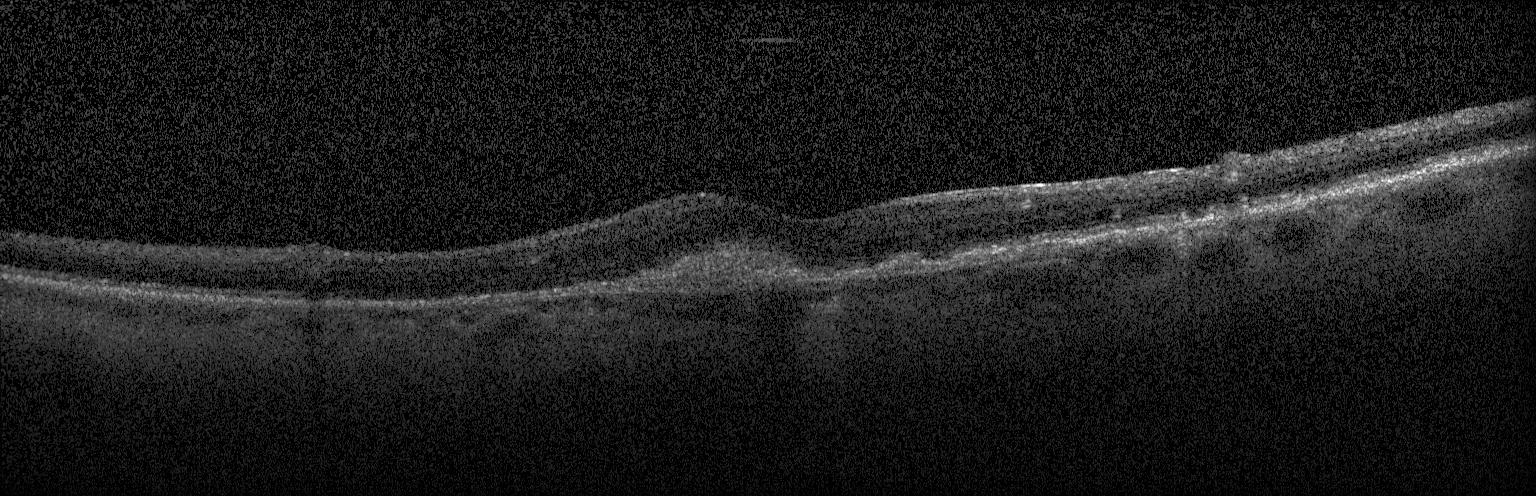

Instrument: Heidelberg Spectralis; spectral-domain OCT; through the macula; OCT B-scan — Assessment: CNV.